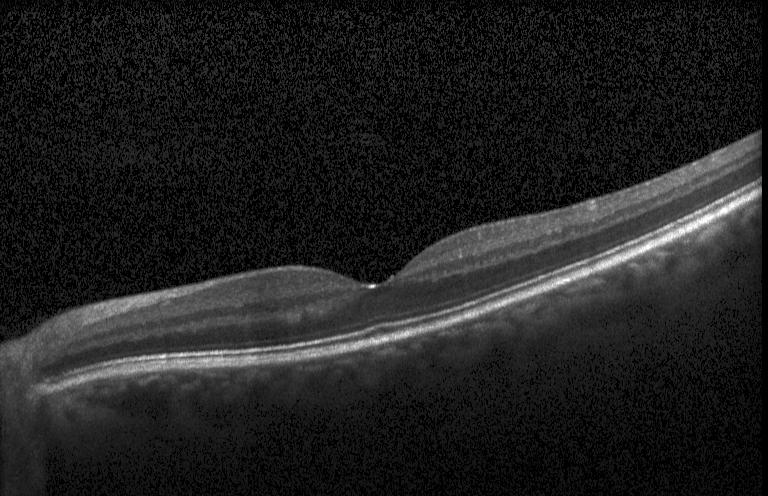
This B-scan demonstrates no choroidal neovascularization, diabetic macular edema, or drusen.